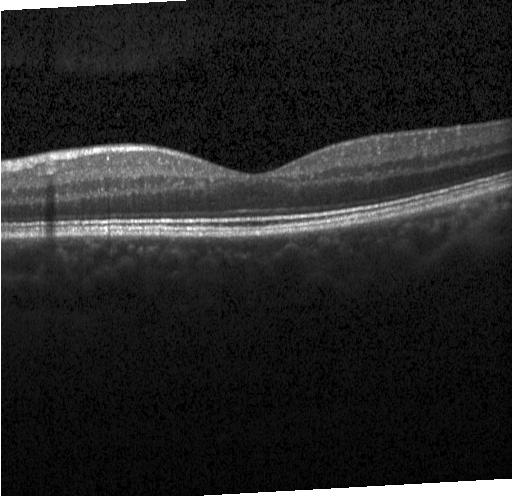 Optical coherence tomography scan. SD-OCT. Heidelberg Spectralis
Finding: no choroidal neovascularization, no diabetic macular edema, and no drusen.